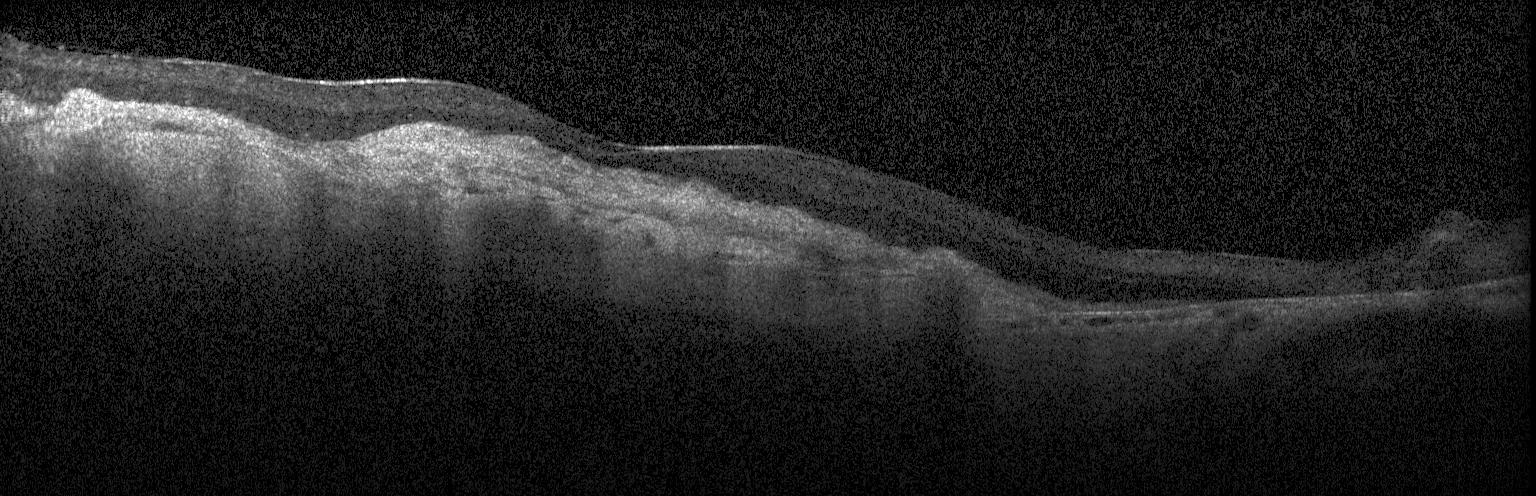 Finding: CNV.